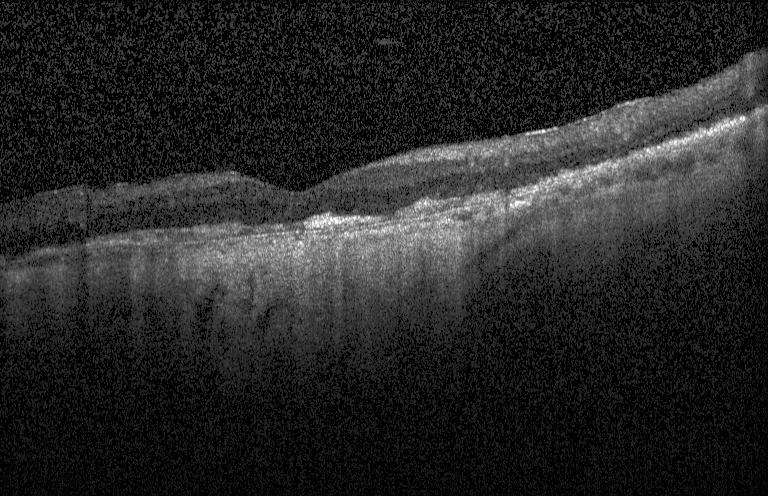 OCT B-scan; SD-OCT; macular scan.
The scan shows a choroidal neovascular membrane.